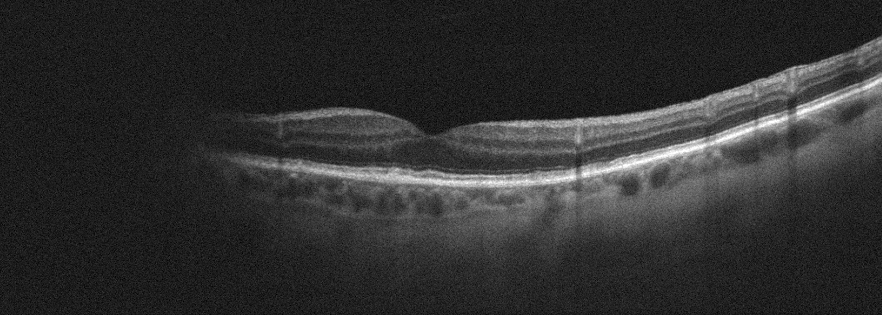 Retinal OCT B-scan · left eye. OCT finding: age-related macular degeneration (AMD).